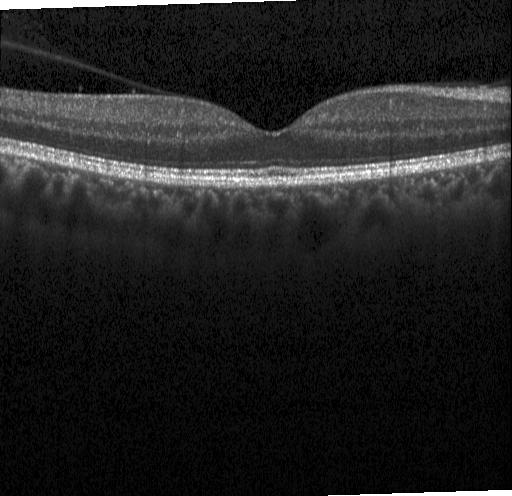

Macular scan · spectral-domain OCT · OCT line scan
Assessment: no CNV, DME, or drusen.